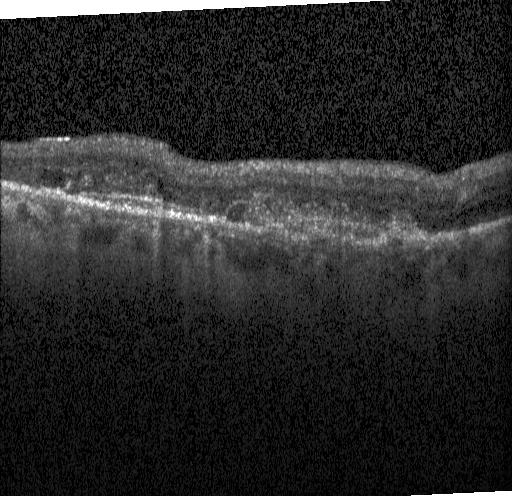 Spectral-domain optical coherence tomography; optical coherence tomography scan; instrument: Heidelberg Spectralis; macular scan. OCT finding: a choroidal neovascular membrane.